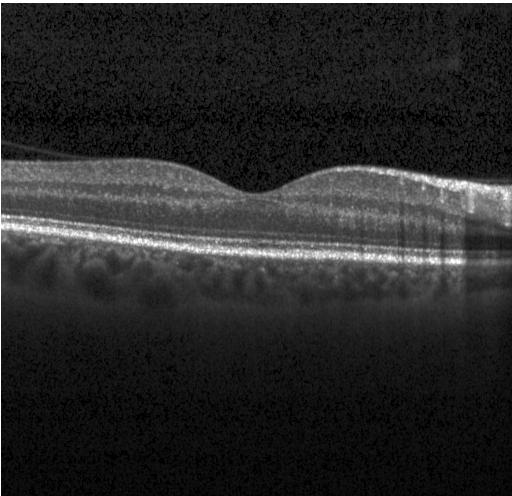
OCT B-scan. Spectral-domain OCT
Dx: no choroidal neovascularization, diabetic macular edema, or drusen.